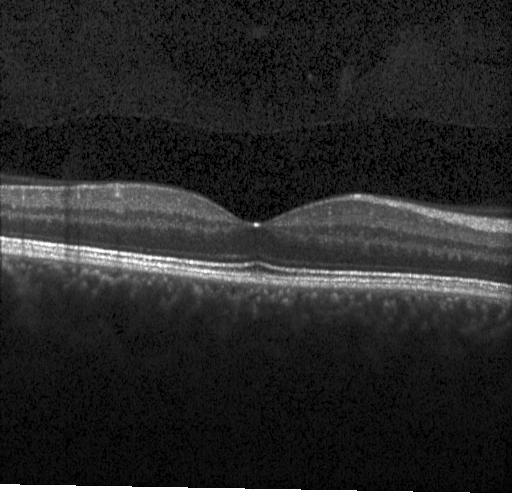

Optical coherence tomography B-scan — Finding: no evidence of choroidal neovascularization, diabetic macular edema, or drusen.